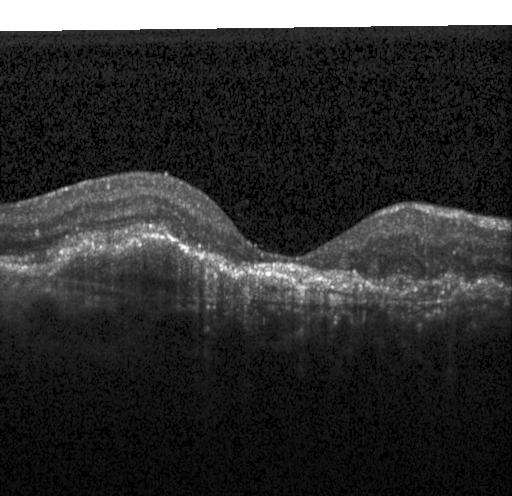

OCT B-scan
Diagnosis: a choroidal neovascular membrane.